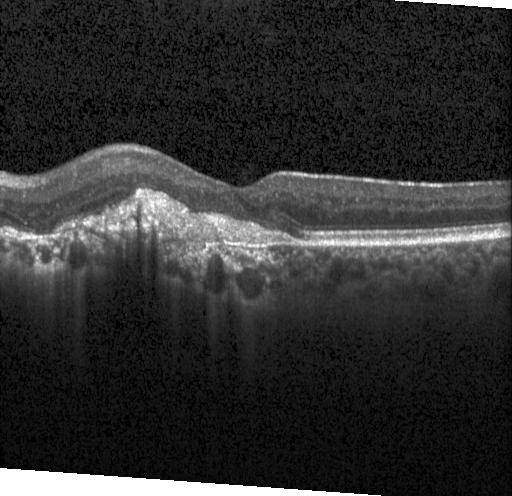

Impression: choroidal neovascularization (CNV).